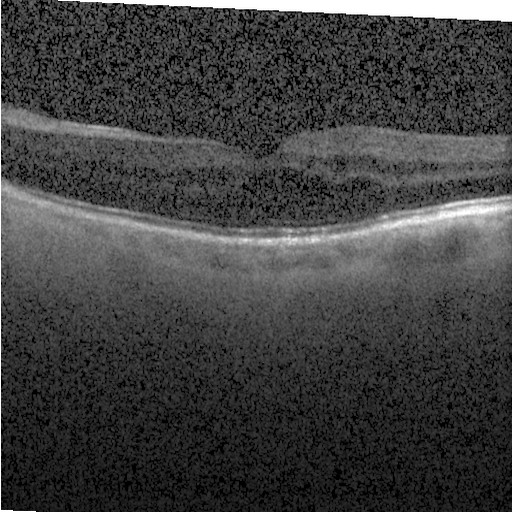 Retinal OCT cross-section. Diagnosis: diabetic macular edema.